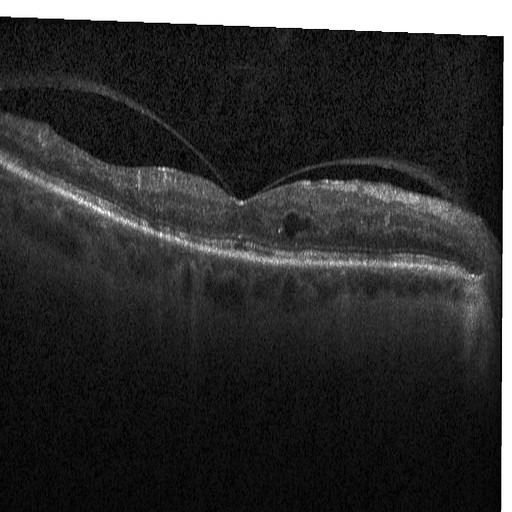
OCT scan showing diabetic macular edema (DME).